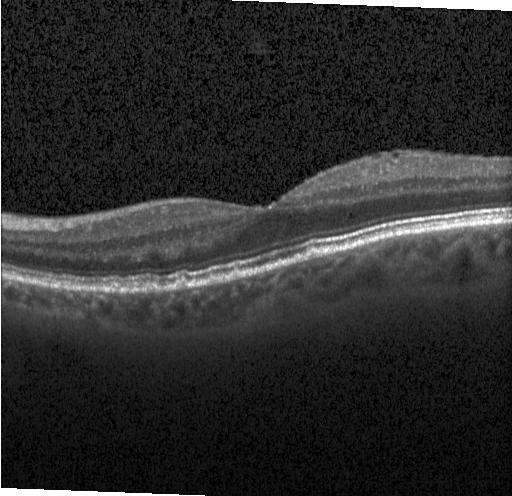 Retinal OCT cross-section
Macular OCT: sub-RPE drusenoid deposits.